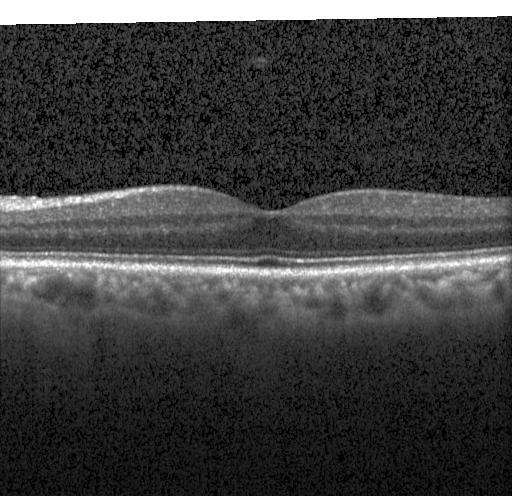
Fovea-centered, retinal OCT B-scan, SD-OCT, Heidelberg Spectralis — Diagnosis: no CNV, no DME, and no drusen.